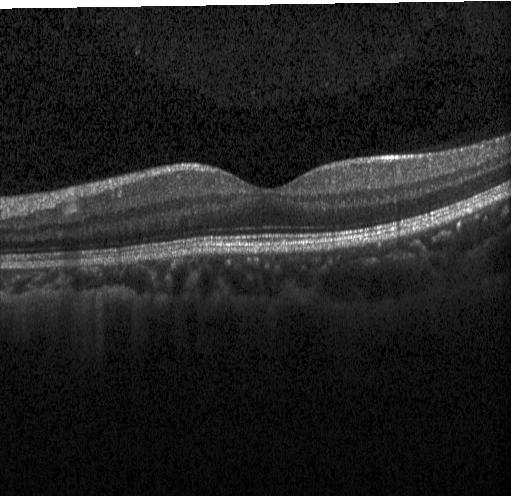
Centered on the fovea; retinal OCT B-scan; spectral-domain OCT.
Impression: no choroidal neovascularization, diabetic macular edema, or drusen.